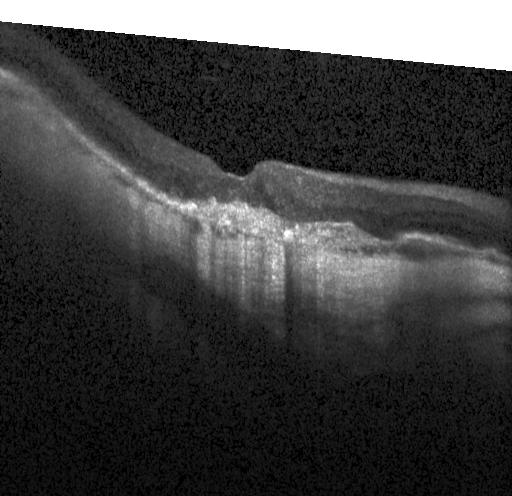

Dx: a choroidal neovascular membrane.